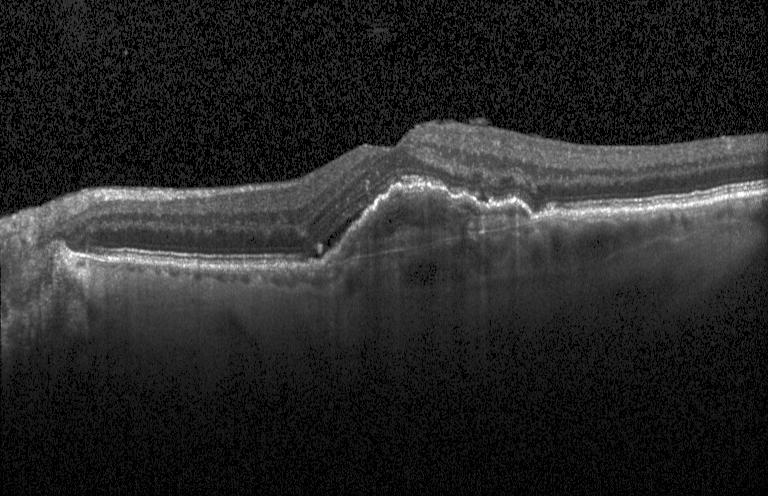
Finding: a choroidal neovascular membrane.